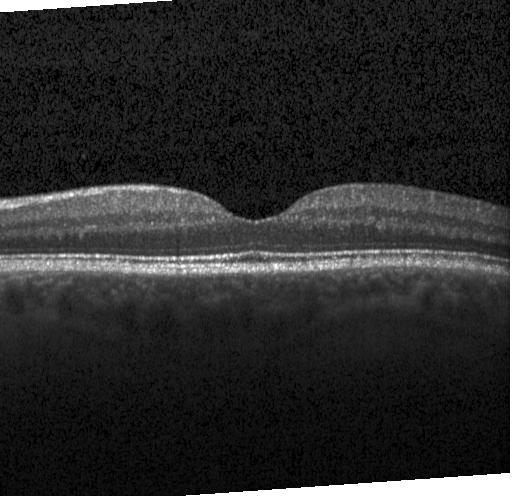

Spectral-domain optical coherence tomography; fovea-centered; Heidelberg Spectralis; OCT line scan.
OCT finding: no CNV, no DME, and no drusen.